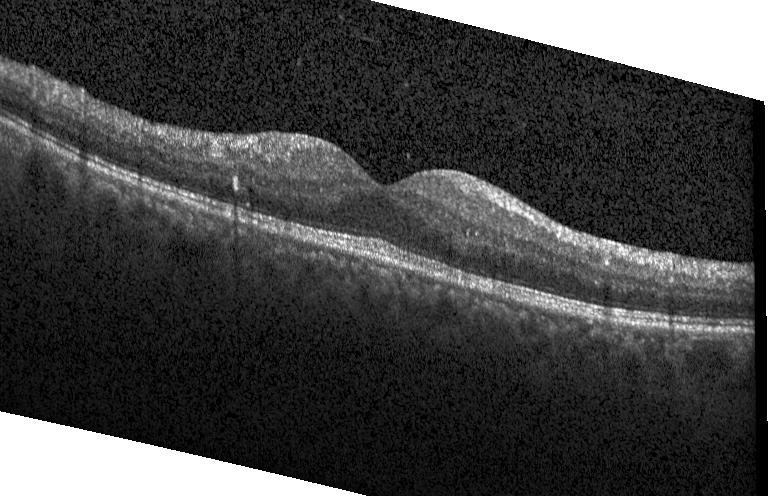
Impression: neither choroidal neovascularization, diabetic macular edema, nor drusen.